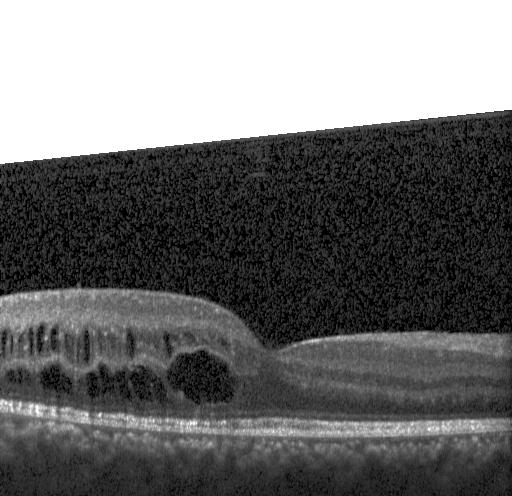

Macular scan · SD-OCT · optical coherence tomography scan. The scan shows diabetic macular edema (DME).